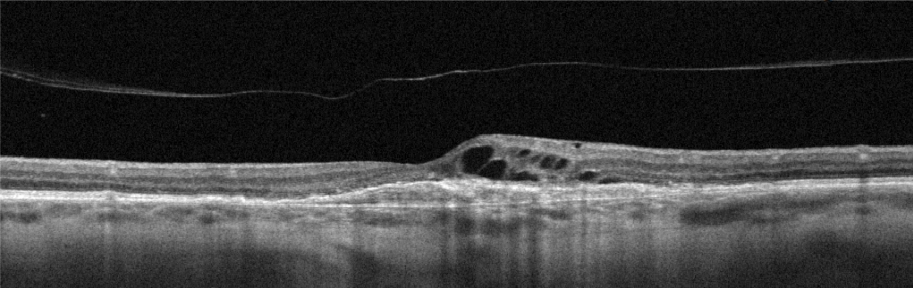
OCT B-scan showing age-related macular degeneration.